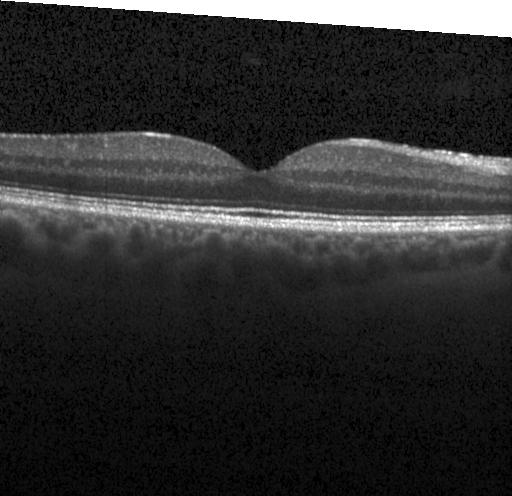 Instrument: Heidelberg Spectralis, through the macula, OCT B-scan, SD-OCT — Diagnosis: no choroidal neovascularization, diabetic macular edema, or drusen.